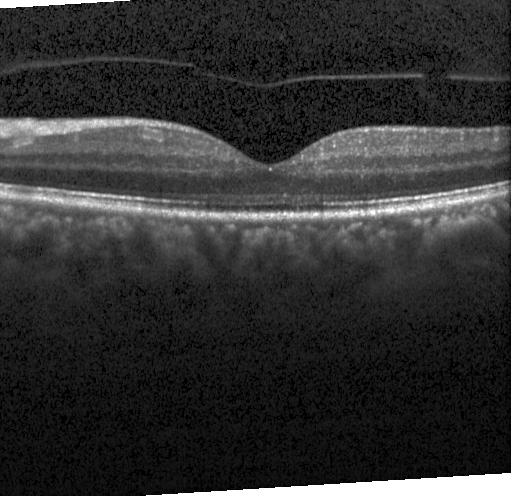

Through the macula, optical coherence tomography scan. Assessment: neither CNV, DME, nor drusen.